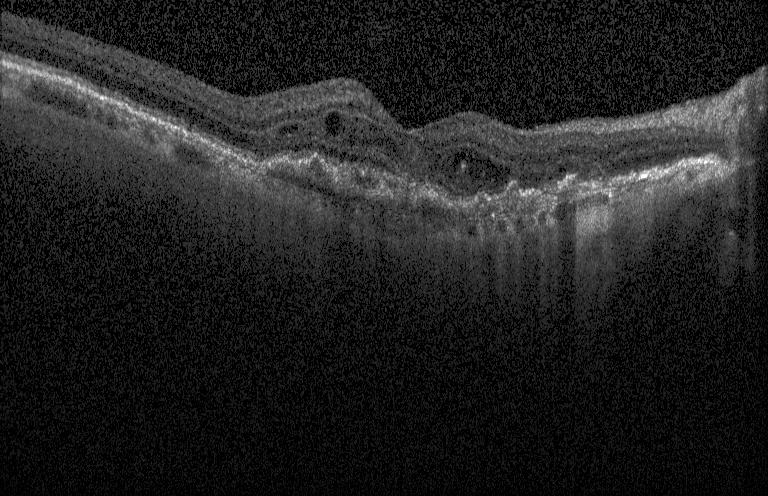
Retinal OCT cross-section
The scan shows choroidal neovascularization.